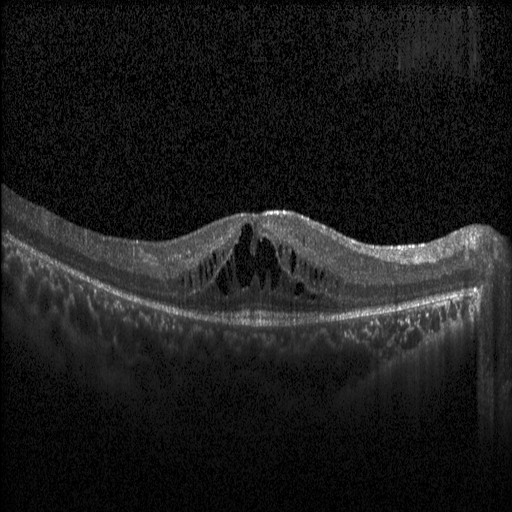

Spectral-domain optical coherence tomography · OCT B-scan. Finding: DME.